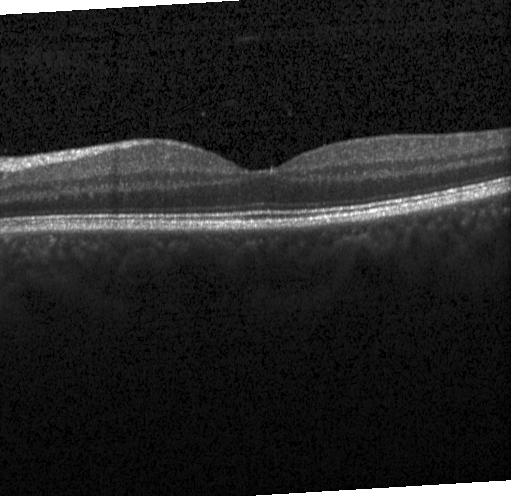

Finding: no evidence of choroidal neovascularization, diabetic macular edema, or drusen.